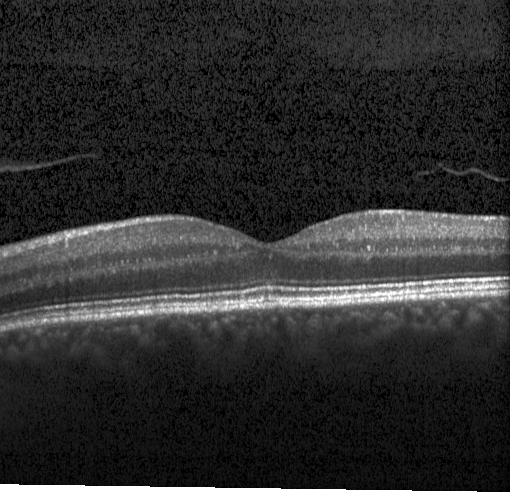 Horizontal scan through the fovea, optical coherence tomography B-scan, Heidelberg Spectralis OCT system
Dx: no choroidal neovascularization, diabetic macular edema, or drusen.